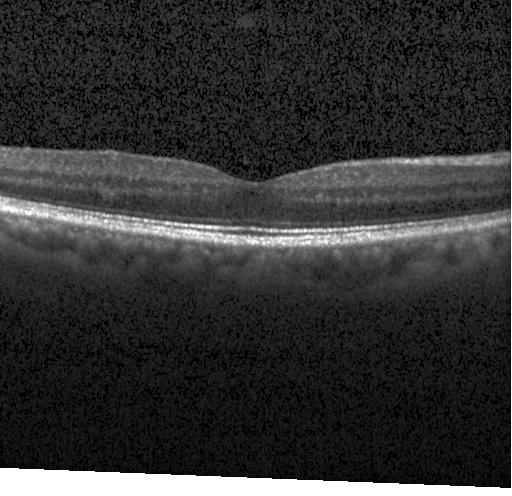 Spectral-domain OCT, OCT line scan, Heidelberg Spectralis OCT system
Diagnosis: no CNV, DME, or drusen.